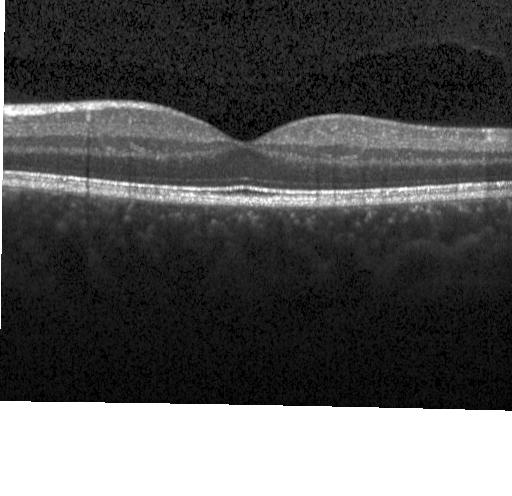
Macular OCT demonstrating no evidence of choroidal neovascularization, diabetic macular edema, or drusen.